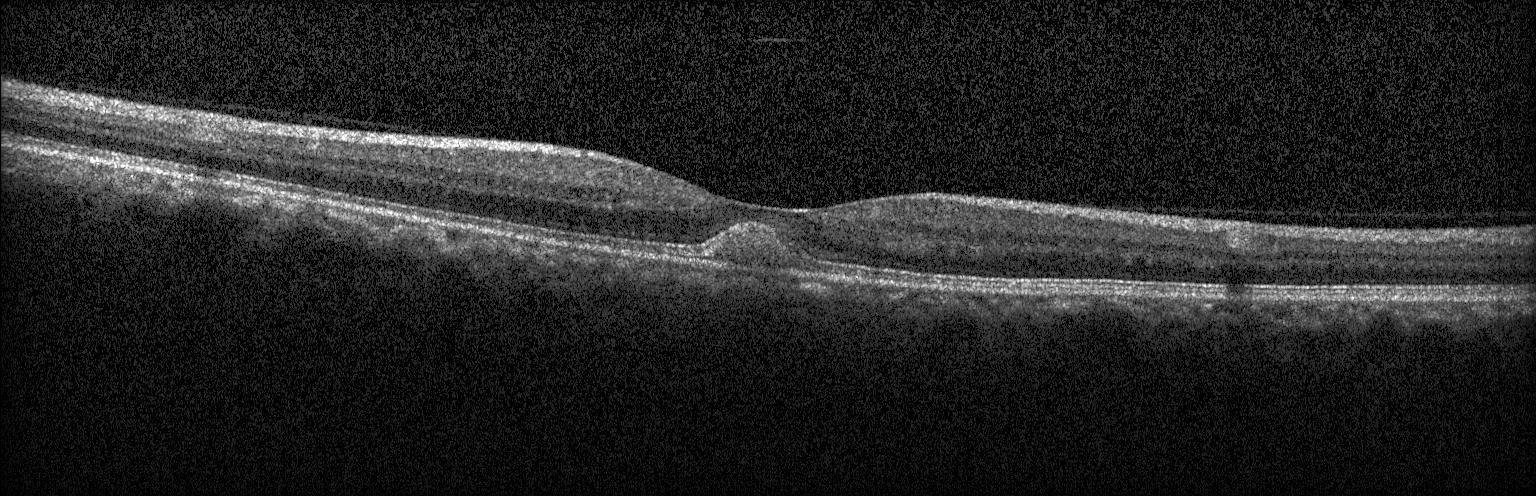 Impression: CNV.